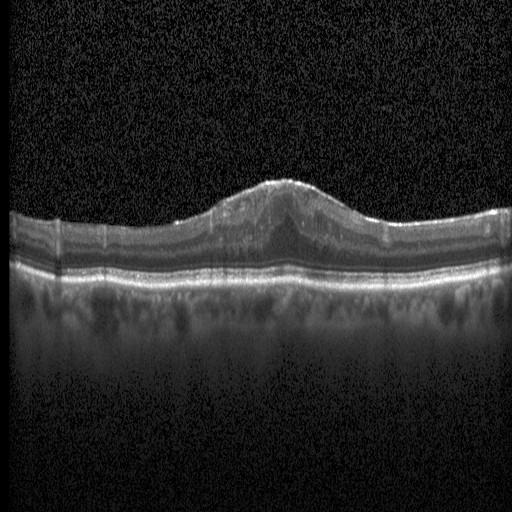
Macular OCT demonstrating diabetic macular edema.